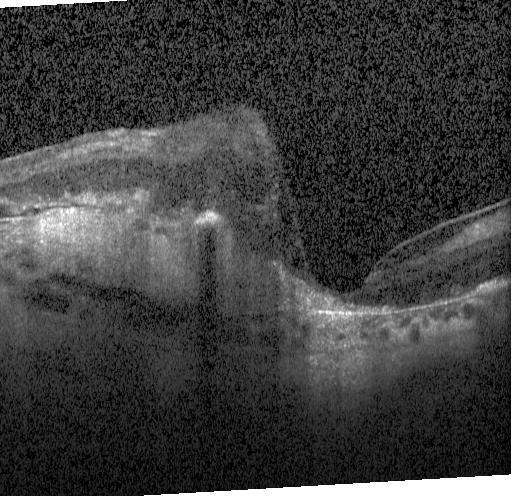 Macular OCT: a choroidal neovascular membrane.